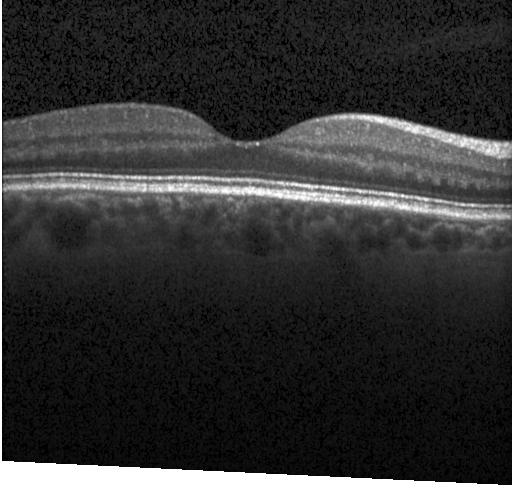
OCT B-scan, SD-OCT — The scan shows neither choroidal neovascularization, diabetic macular edema, nor drusen.